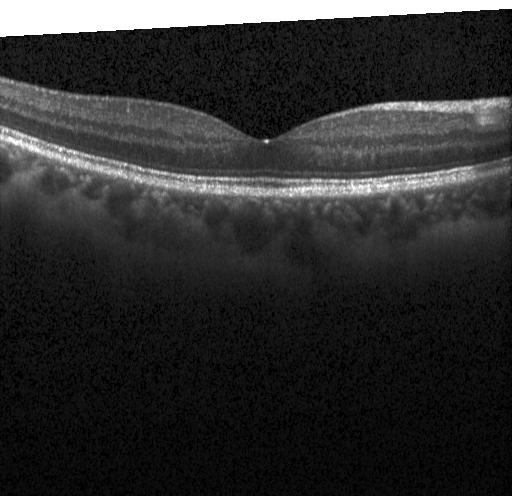
SD-OCT, acquired on a Heidelberg Spectralis, optical coherence tomography B-scan.
OCT finding: no evidence of choroidal neovascularization, diabetic macular edema, or drusen.